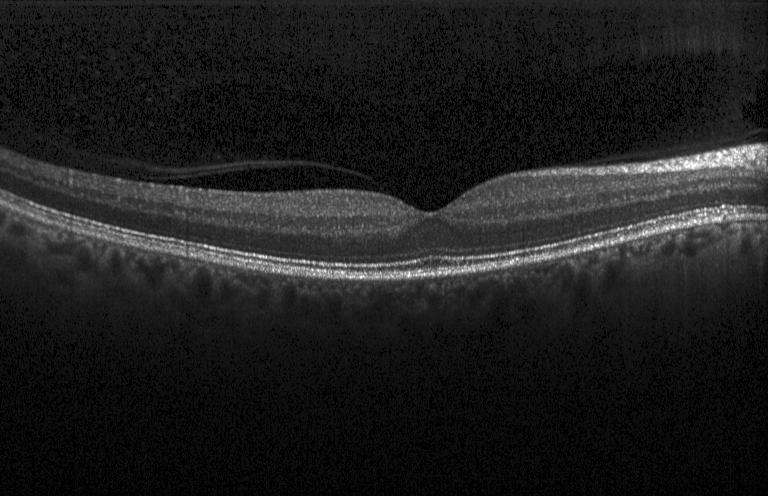

Retinal OCT B-scan — Impression: neither CNV, DME, nor drusen.